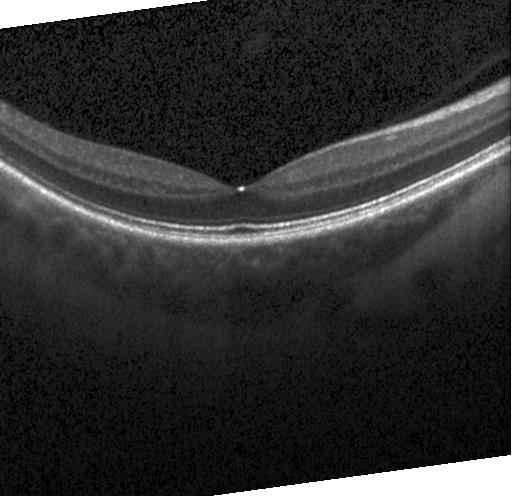

Spectral-domain OCT, optical coherence tomography scan
Impression: no evidence of choroidal neovascularization, diabetic macular edema, or drusen.